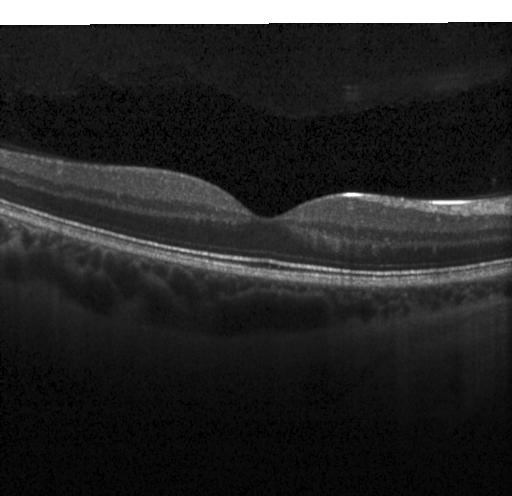 Finding: no choroidal neovascularization, diabetic macular edema, or drusen.